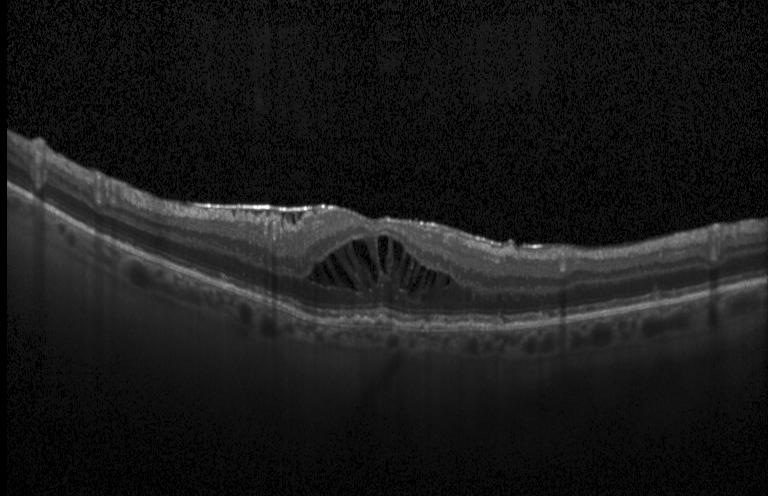 Retinal OCT B-scan
Dx: DME.